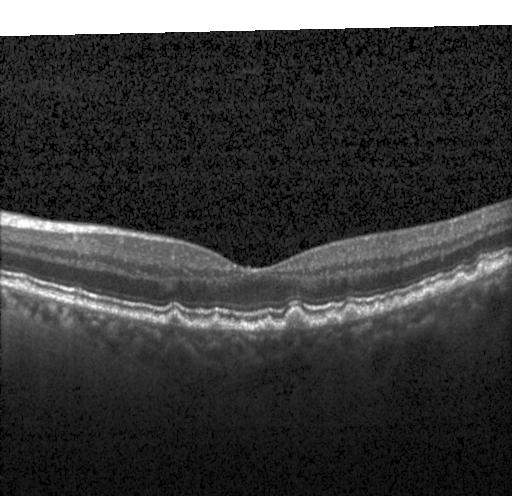
Optical coherence tomography scan; through the macula; SD-OCT; acquired on a Heidelberg Spectralis — Impression: sub-RPE drusenoid deposits.